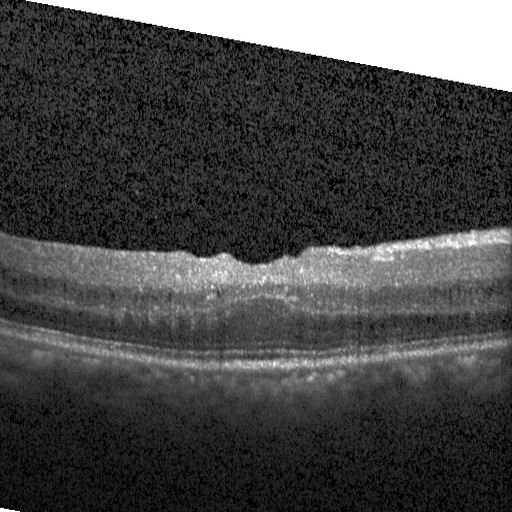

Optical coherence tomography scan
Impression: DME.